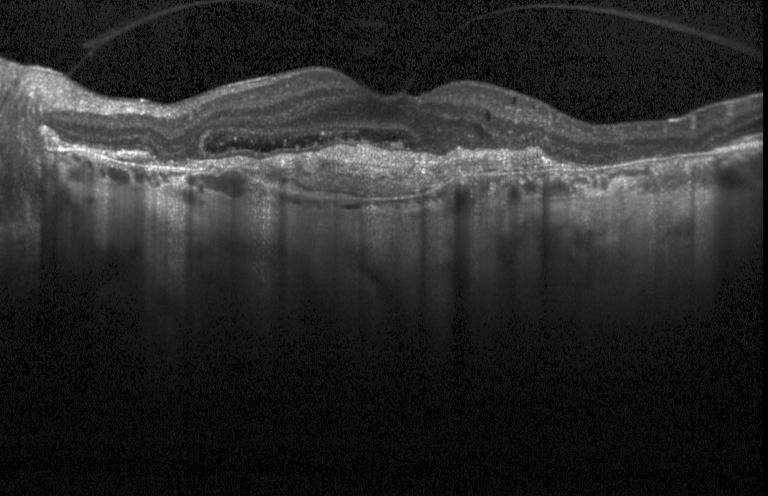

OCT line scan · acquired on a Heidelberg Spectralis. OCT finding: choroidal neovascularization.